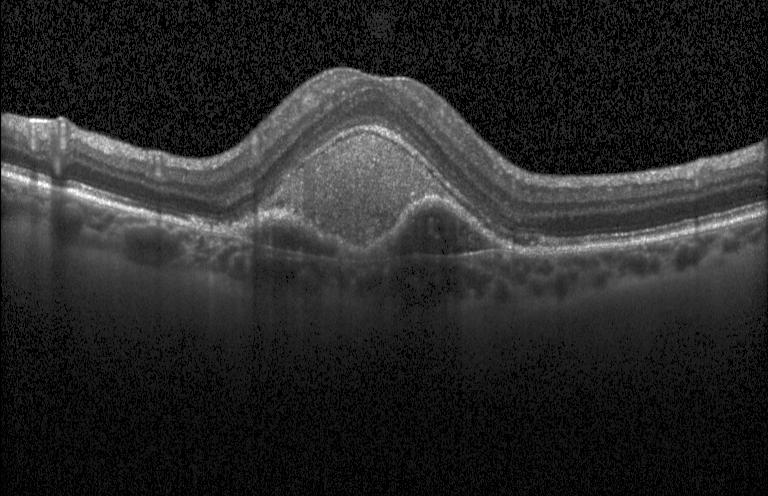

Retinal OCT B-scan — Assessment: a choroidal neovascular membrane.